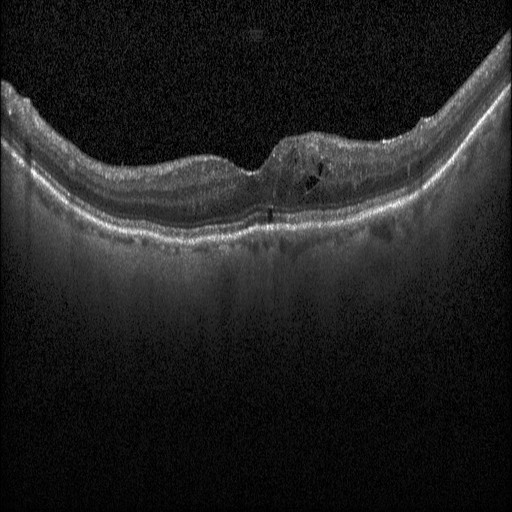
Finding: diabetic macular edema.